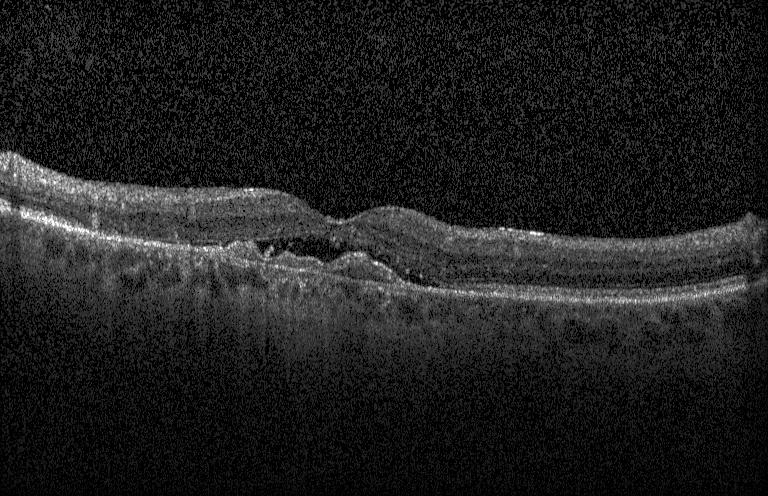

Retinal OCT B-scan.
Impression: CNV.